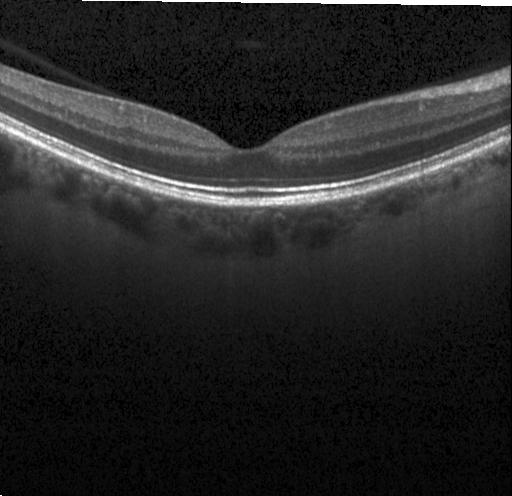
Centered on the fovea; retinal OCT B-scan
Diagnosis: neither choroidal neovascularization, diabetic macular edema, nor drusen.